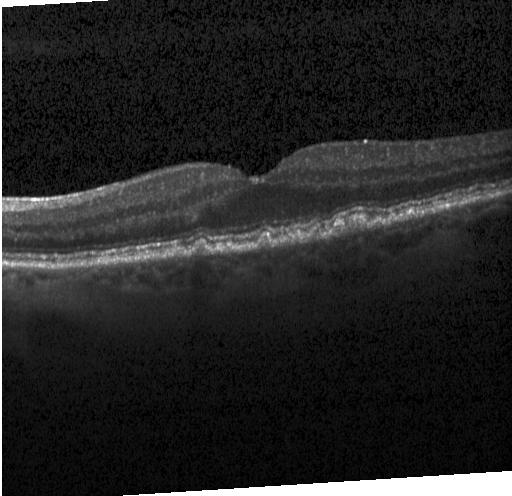

Impression: multiple drusen.